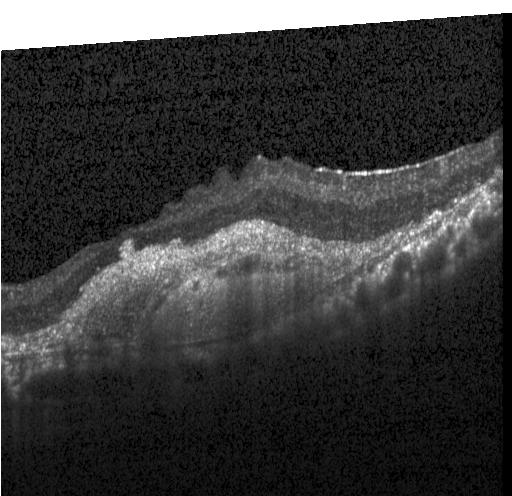 Finding: a choroidal neovascular membrane.